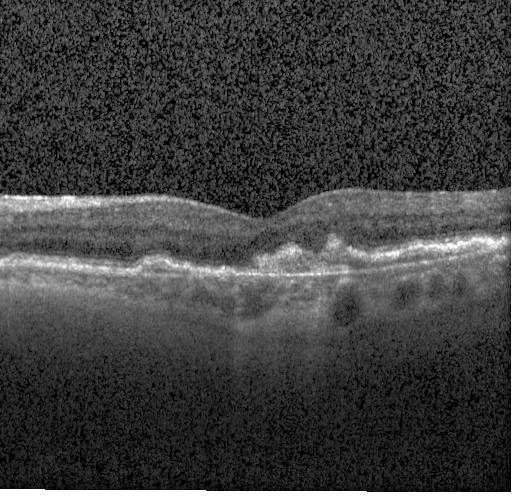
OCT line scan, Heidelberg Spectralis
Finding: a choroidal neovascular membrane.